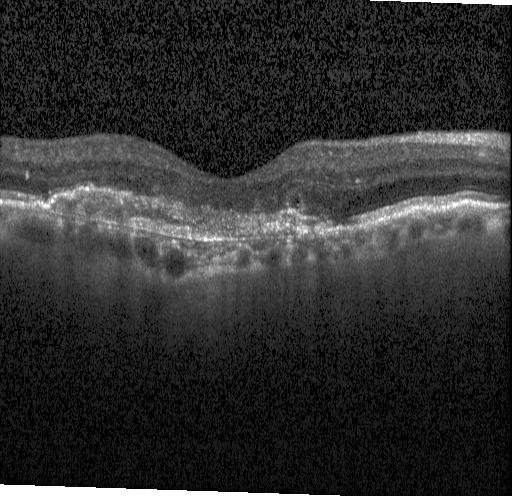

Dx: choroidal neovascularization (CNV).